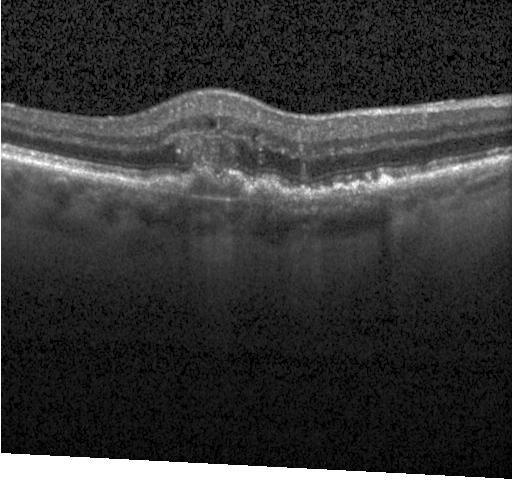

Spectral-domain OCT. Retinal OCT cross-section. This B-scan demonstrates choroidal neovascularization (CNV).